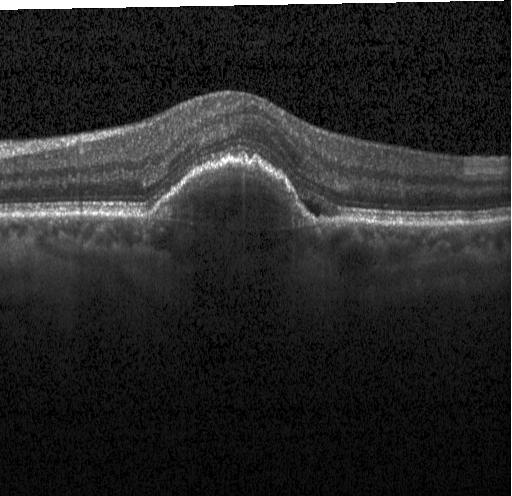 Impression: a choroidal neovascular membrane.